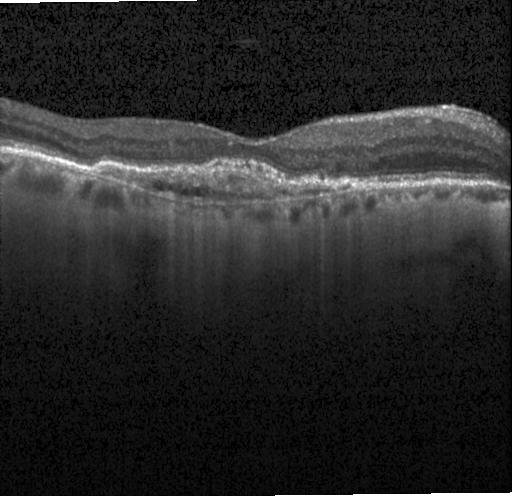 OCT finding: CNV.